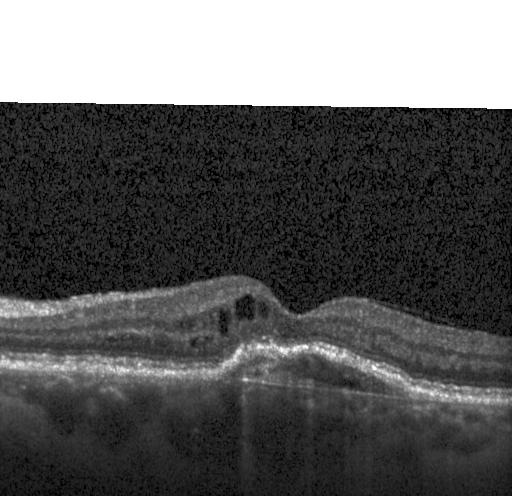 Retinal OCT cross-section showing choroidal neovascularization.